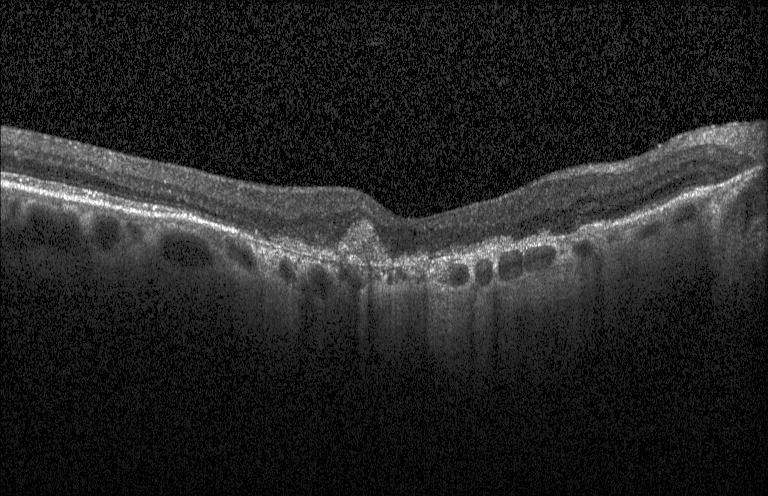
OCT finding: choroidal neovascularization.